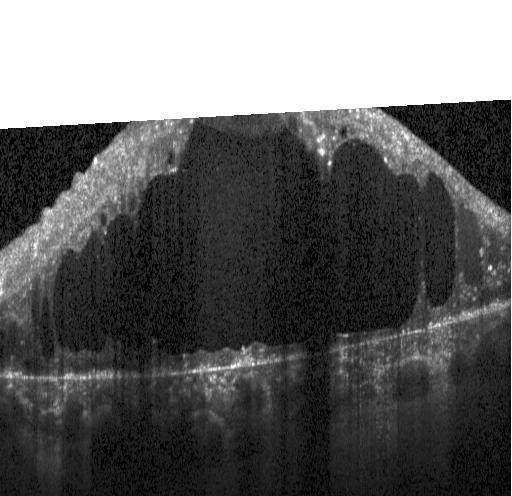 Spectral-domain OCT. Through the macula. Optical coherence tomography scan.
DME.